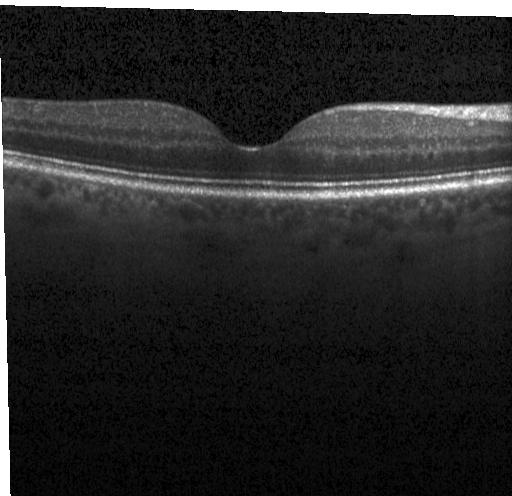
Optical coherence tomography B-scan. Through the macula. Heidelberg Spectralis. Spectral-domain OCT. Macular OCT: neither choroidal neovascularization, diabetic macular edema, nor drusen.